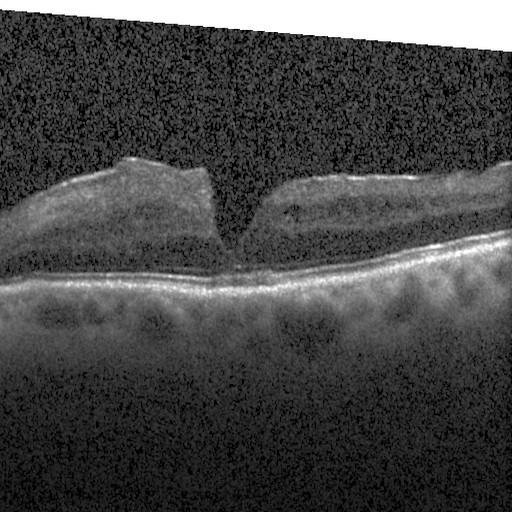 OCT B-scan showing DME.